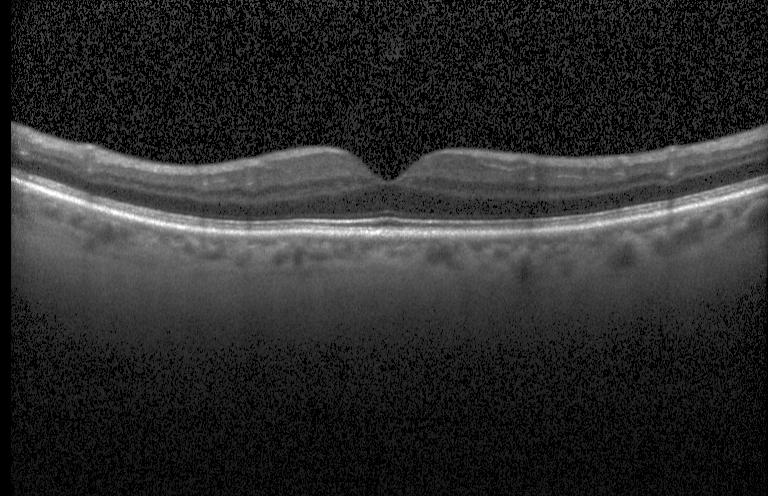
Dx: no choroidal neovascularization, no diabetic macular edema, and no drusen.